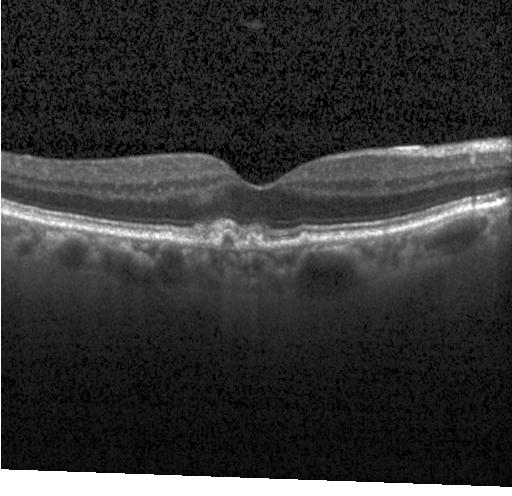 Spectral-domain optical coherence tomography. Optical coherence tomography B-scan. Diagnosis: drusen.